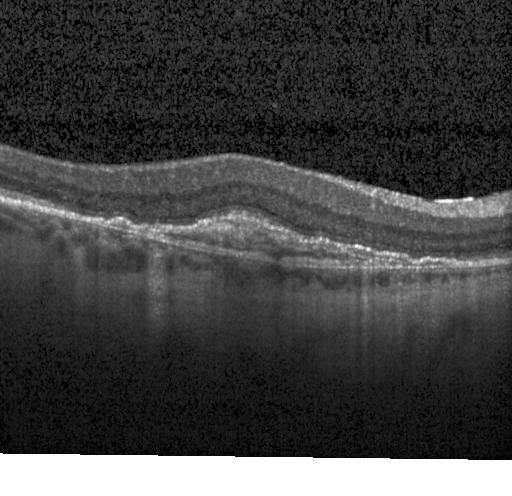
Finding: a choroidal neovascular membrane.